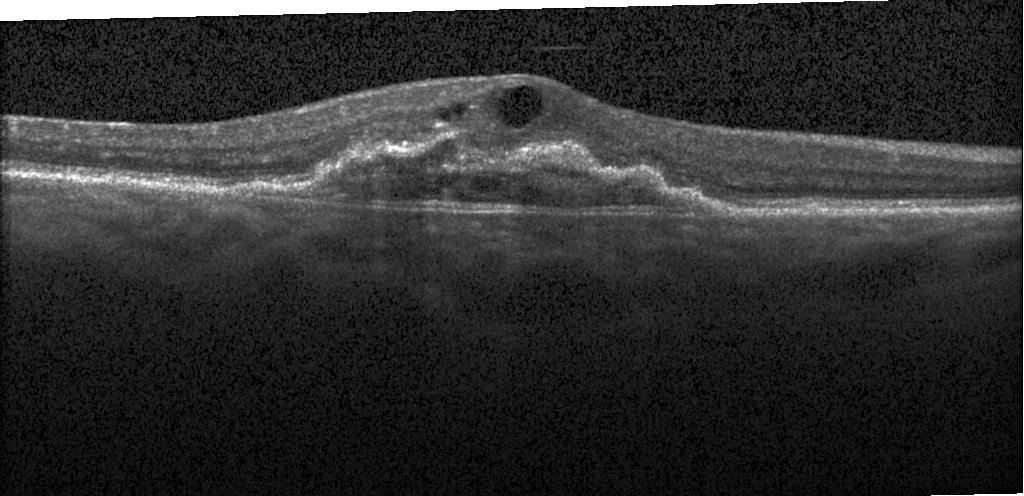
Diagnosis: choroidal neovascularization (CNV).